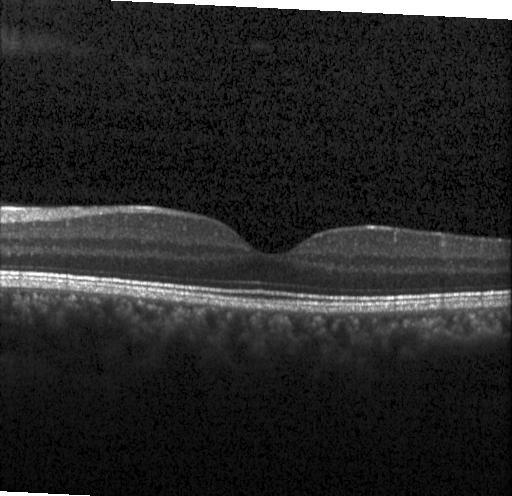 Retinal OCT cross-section, spectral-domain optical coherence tomography, macular scan
Assessment: no CNV, DME, or drusen.